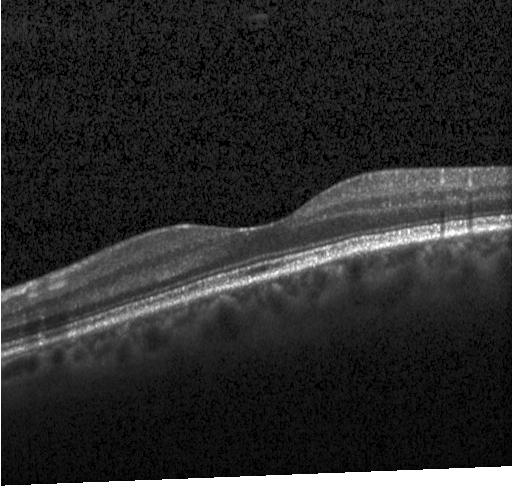 Optical coherence tomography B-scan — Impression: no evidence of choroidal neovascularization, diabetic macular edema, or drusen.